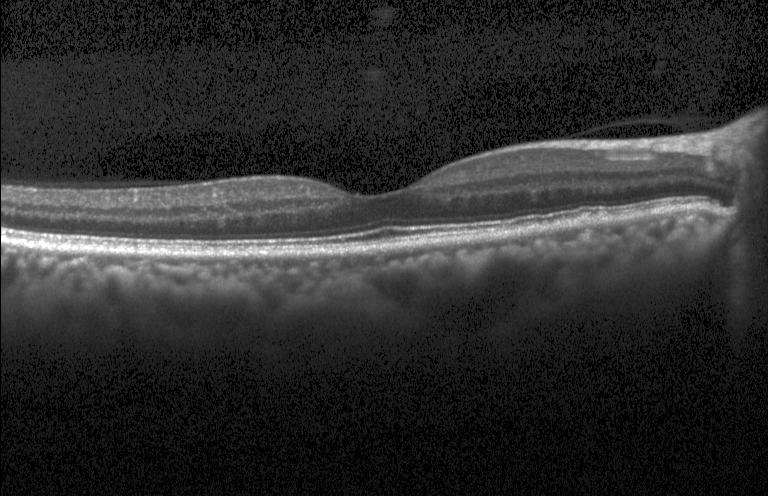
Heidelberg Spectralis OCT system, retinal OCT B-scan
Impression: no CNV, DME, or drusen.